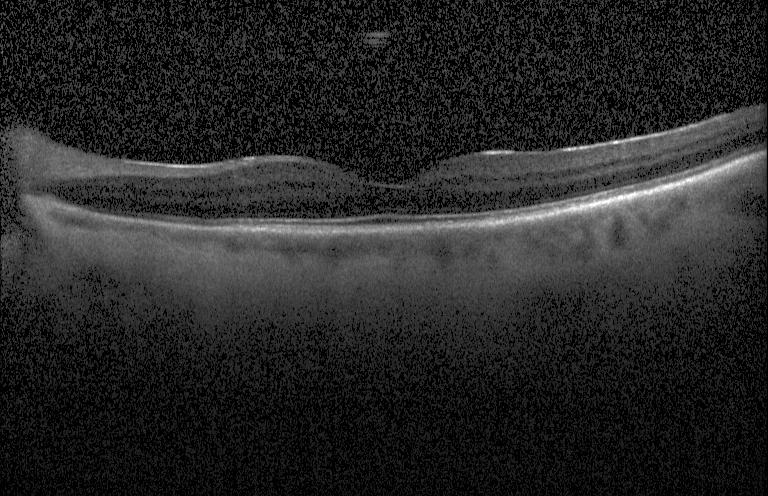
Fovea-centered. Optical coherence tomography B-scan. Spectral-domain OCT — Finding: neither choroidal neovascularization, diabetic macular edema, nor drusen.